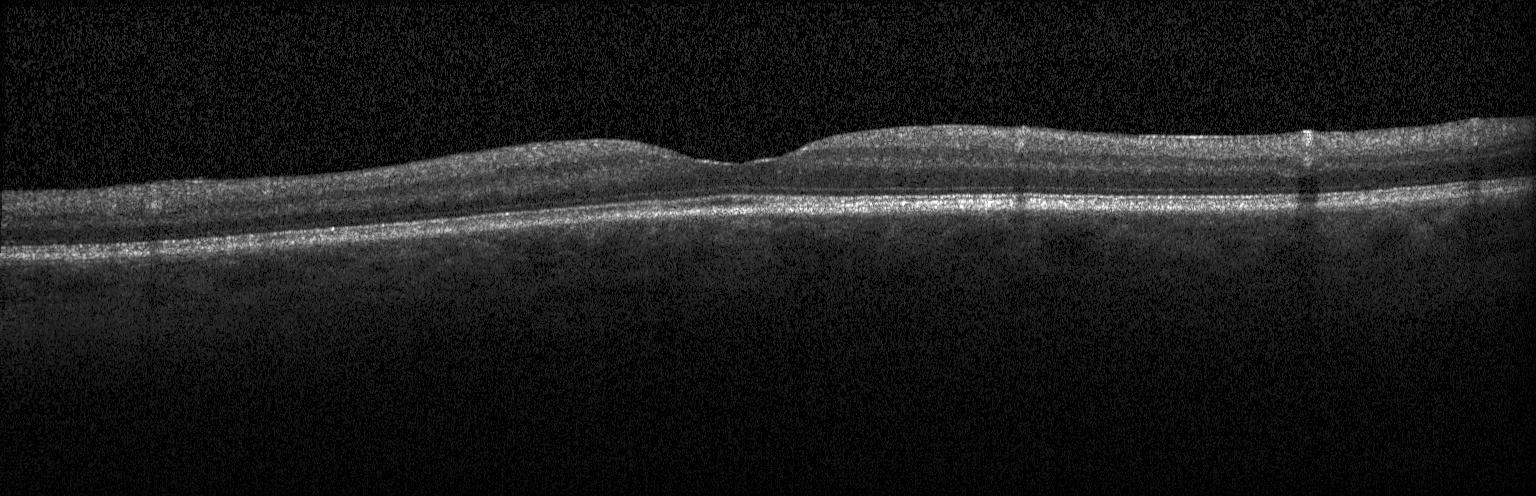 Optical coherence tomography scan. Macular scan. Spectral-domain optical coherence tomography
The scan shows no evidence of CNV, DME, or drusen.